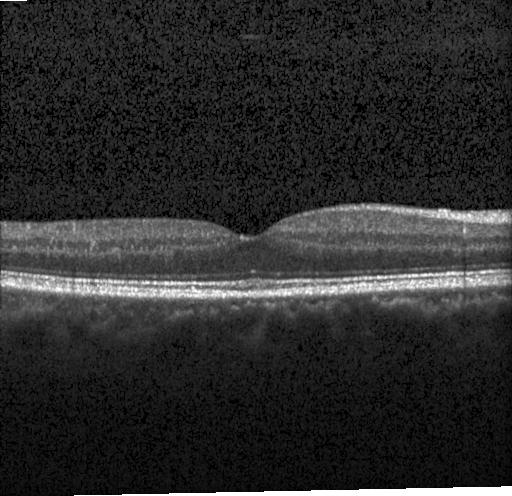 Diagnosis: no CNV, no DME, and no drusen.